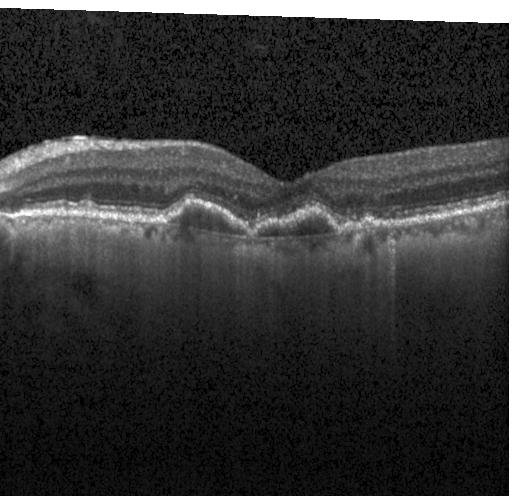 Macular scan; OCT B-scan. The scan shows choroidal neovascularization.